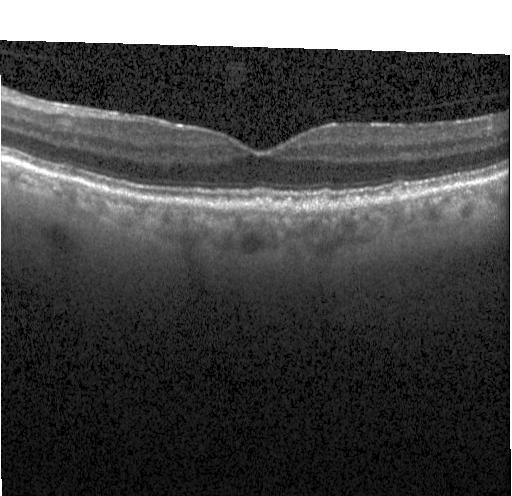

Heidelberg Spectralis OCT system · centered on the fovea · retinal OCT cross-section · spectral-domain optical coherence tomography. Impression: sub-RPE drusenoid deposits.